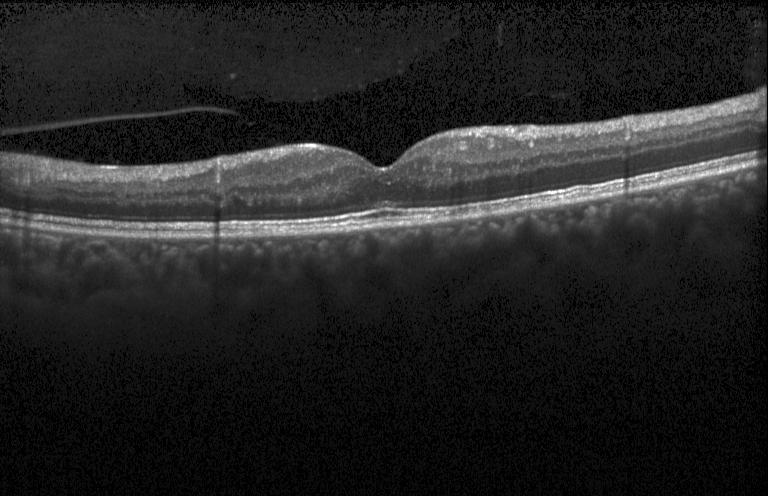
Optical coherence tomography scan.
Finding: no choroidal neovascularization, diabetic macular edema, or drusen.